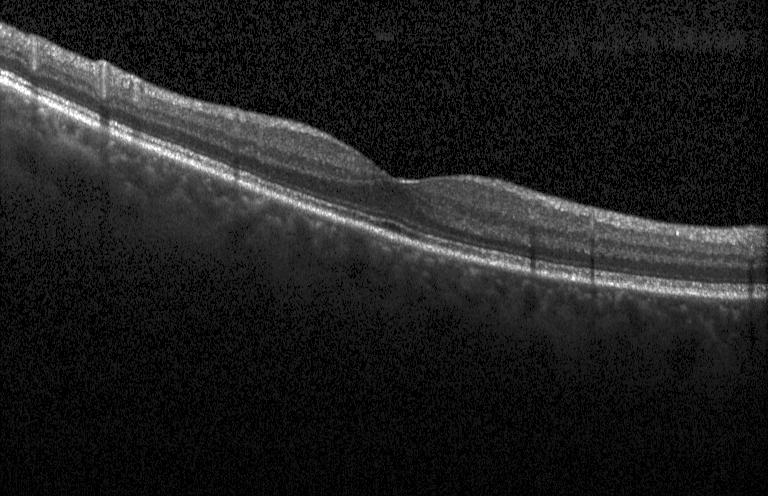
SD-OCT · retinal OCT B-scan · instrument: Heidelberg Spectralis · through the macula
The scan shows no evidence of choroidal neovascularization, diabetic macular edema, or drusen.